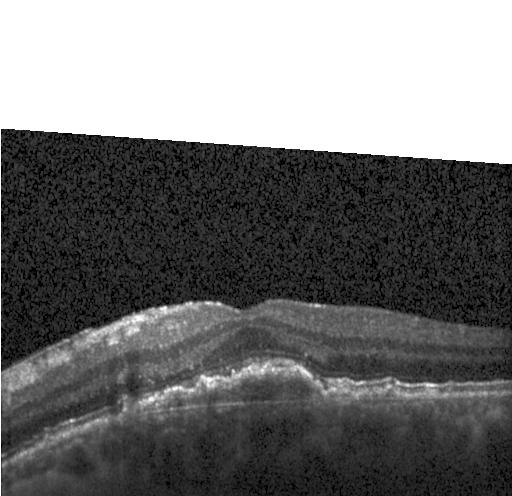

OCT B-scan.
Diagnosis: choroidal neovascularization.